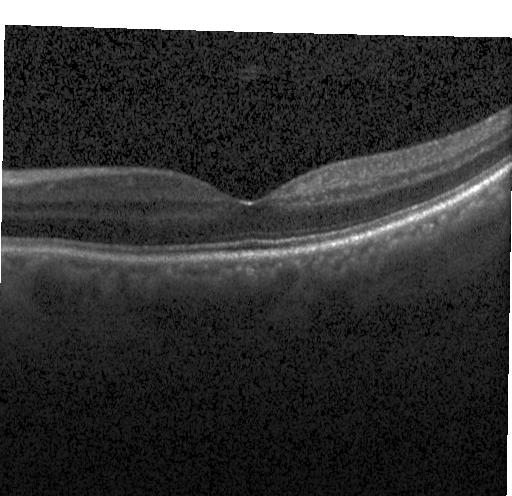
Heidelberg Spectralis · retinal OCT cross-section.
Dx: no evidence of CNV, DME, or drusen.